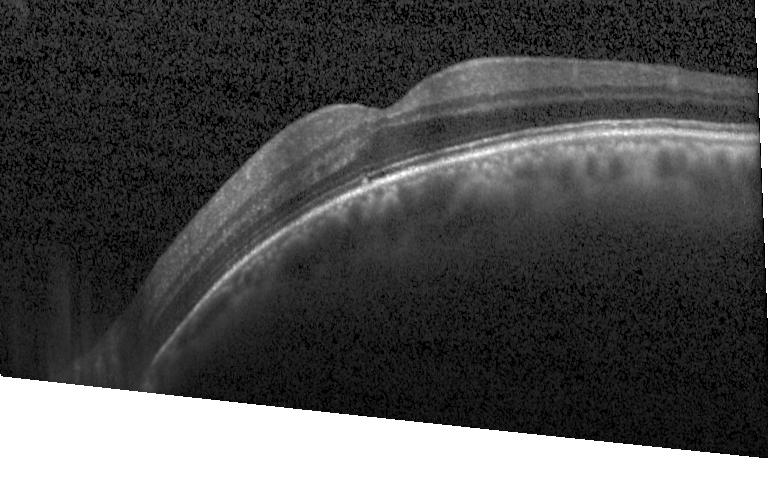
Retinal OCT cross-section. Centered on the fovea — Assessment: no choroidal neovascularization, no diabetic macular edema, and no drusen.